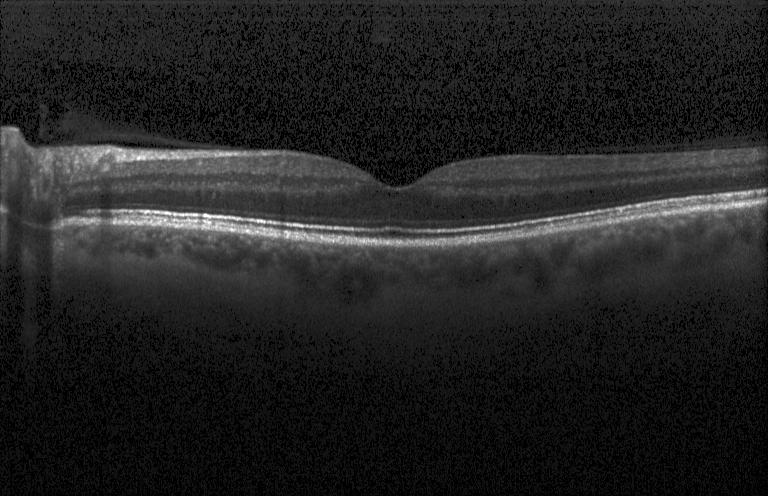
Heidelberg Spectralis OCT system. OCT line scan. Spectral-domain OCT. The scan shows neither choroidal neovascularization, diabetic macular edema, nor drusen.